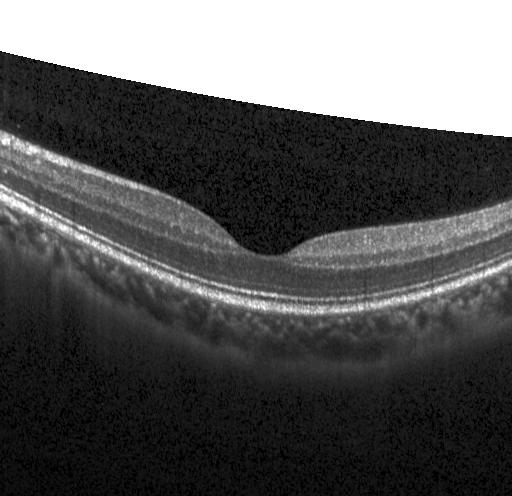
Diagnosis: no evidence of CNV, DME, or drusen.